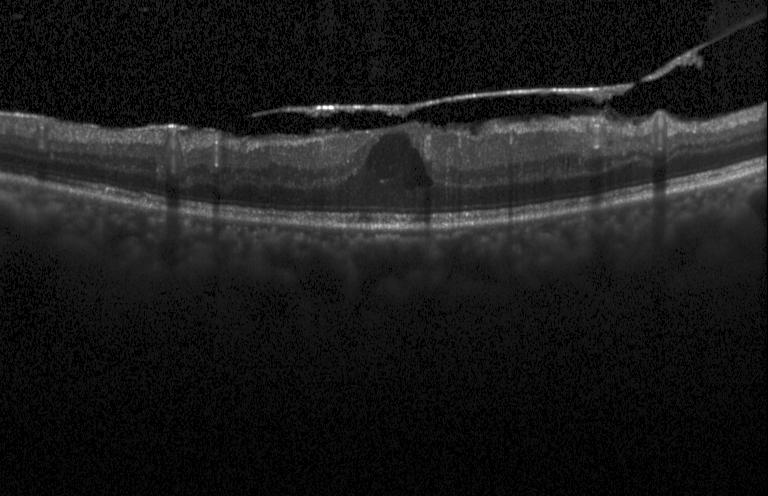 Centered on the fovea, optical coherence tomography B-scan, acquired on a Heidelberg Spectralis. This B-scan demonstrates diabetic macular edema (DME).